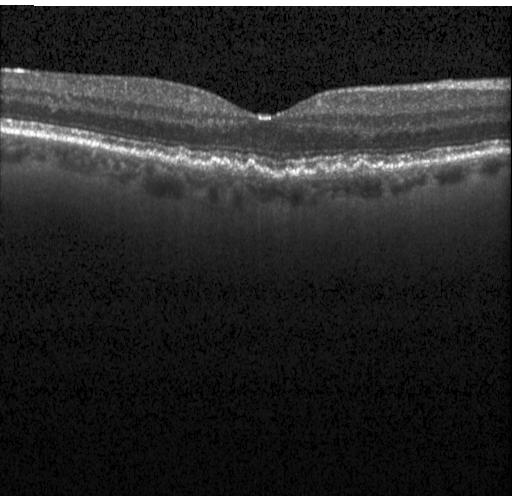
Fovea-centered · acquired on a Heidelberg Spectralis · OCT line scan · spectral-domain optical coherence tomography.
Macular OCT: drusen.